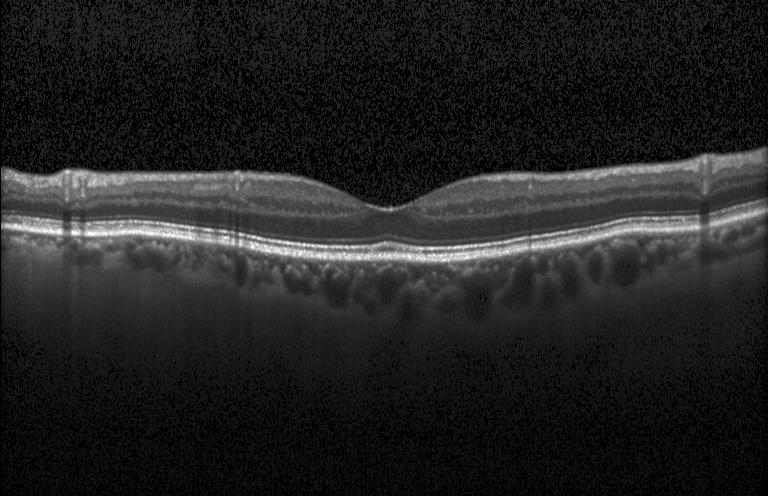

Heidelberg Spectralis, spectral-domain OCT, OCT B-scan, fovea-centered
Macular OCT: no choroidal neovascularization, diabetic macular edema, or drusen.